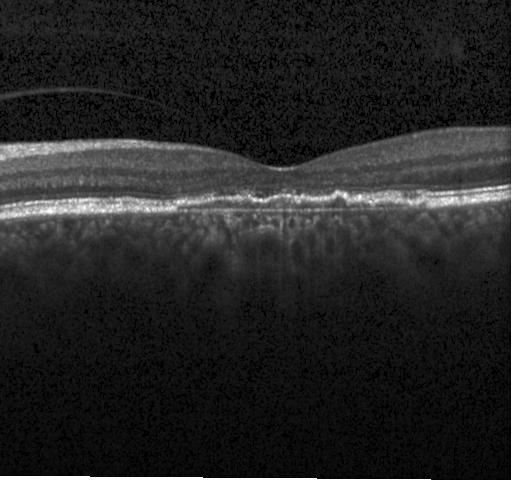 OCT finding: a choroidal neovascular membrane.